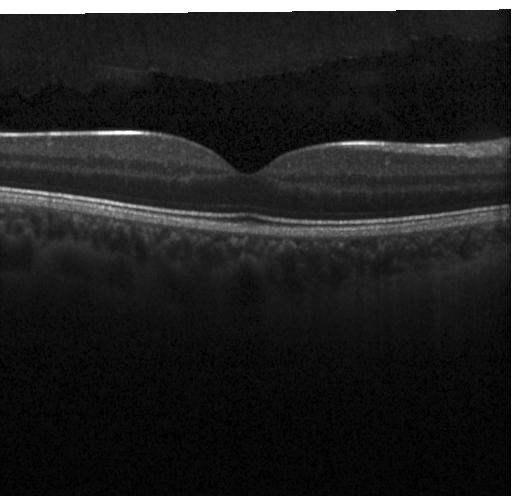 Centered on the fovea, retinal OCT cross-section. Finding: no choroidal neovascularization, diabetic macular edema, or drusen.